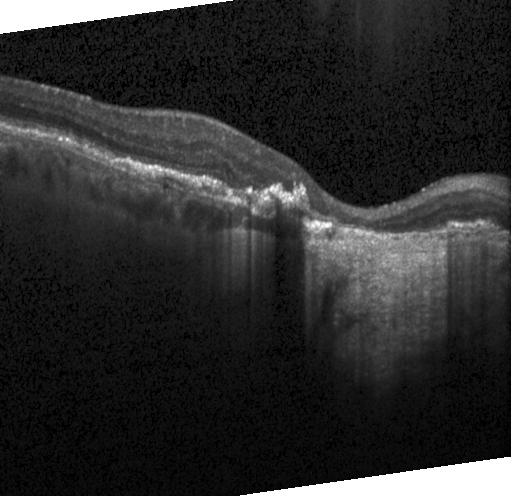
CNV.